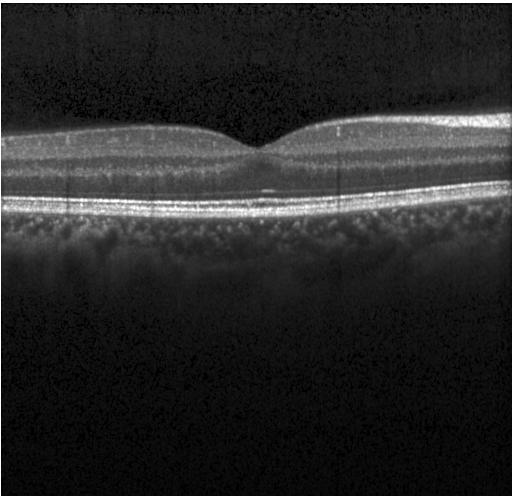

Heidelberg Spectralis, centered on the fovea, OCT B-scan — Diagnosis: no CNV, DME, or drusen.